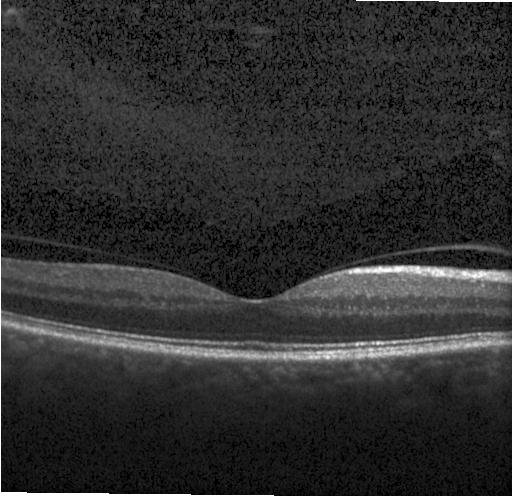 Heidelberg Spectralis; SD-OCT; optical coherence tomography scan.
OCT finding: neither choroidal neovascularization, diabetic macular edema, nor drusen.